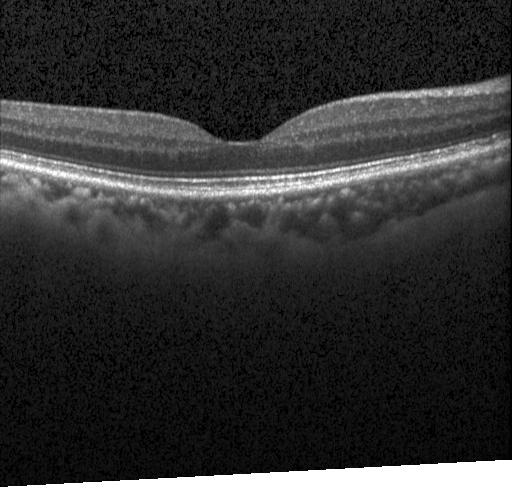 OCT B-scan. Diagnosis: no evidence of choroidal neovascularization, diabetic macular edema, or drusen.